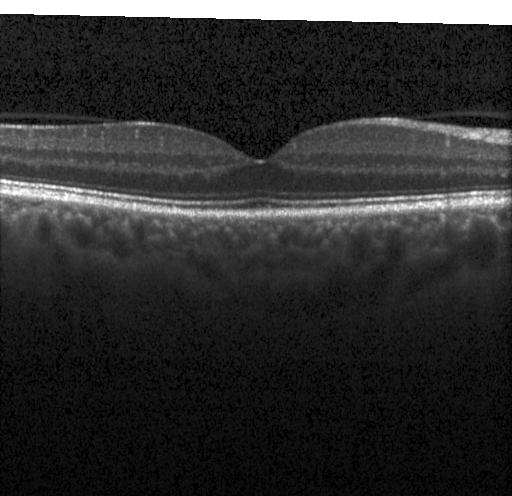

Impression: neither choroidal neovascularization, diabetic macular edema, nor drusen.